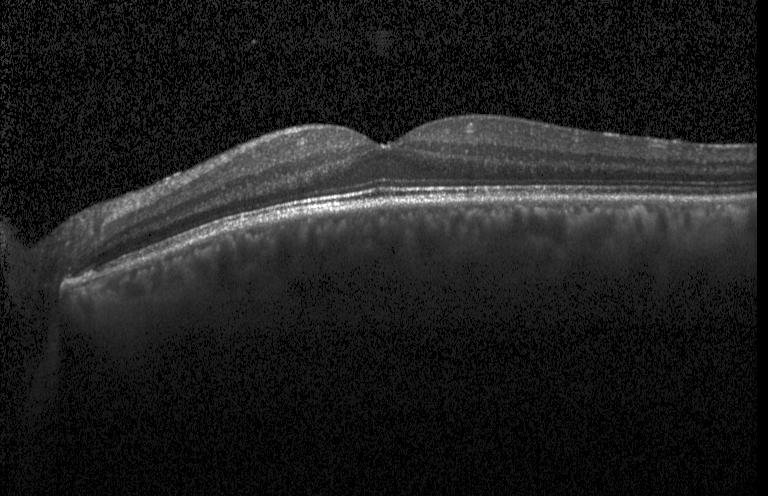

Diagnosis: no CNV, no DME, and no drusen.